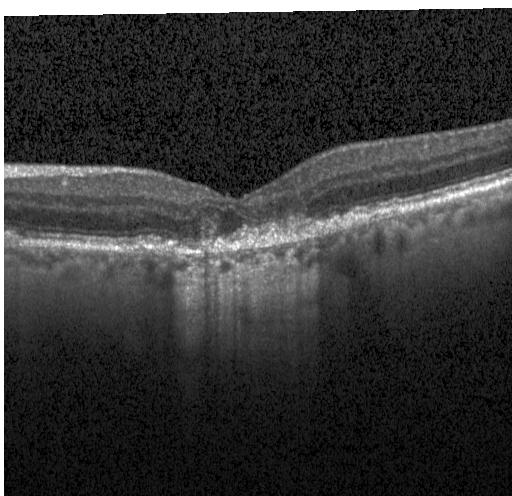 Spectral-domain optical coherence tomography · retinal OCT cross-section
Assessment: a choroidal neovascular membrane.